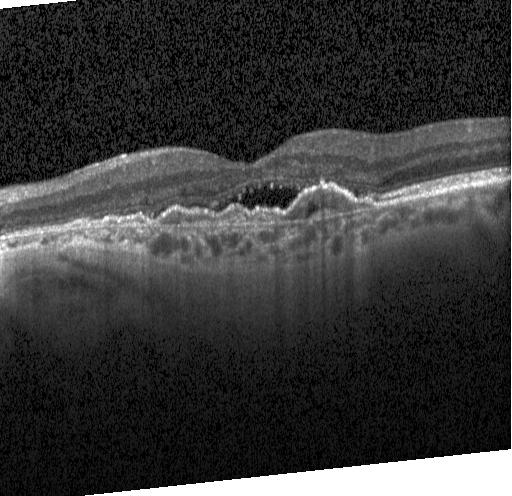

Impression: choroidal neovascularization.